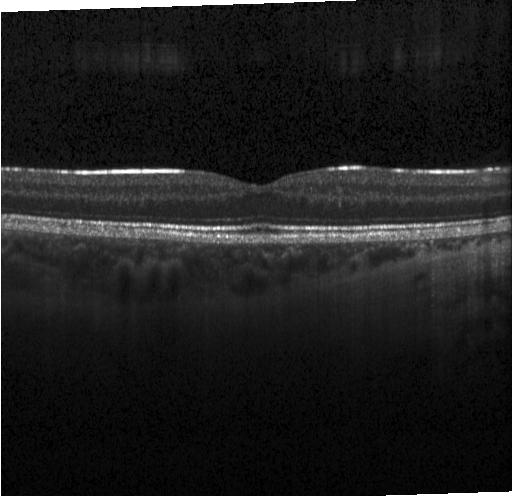

Retinal OCT cross-section. Spectral-domain OCT. Through the macula. No choroidal neovascularization, diabetic macular edema, or drusen.